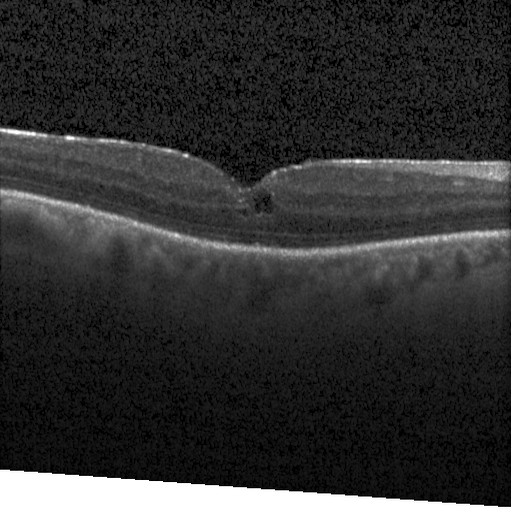

Centered on the fovea; instrument: Heidelberg Spectralis; SD-OCT; OCT B-scan.
Impression: diabetic macular edema.